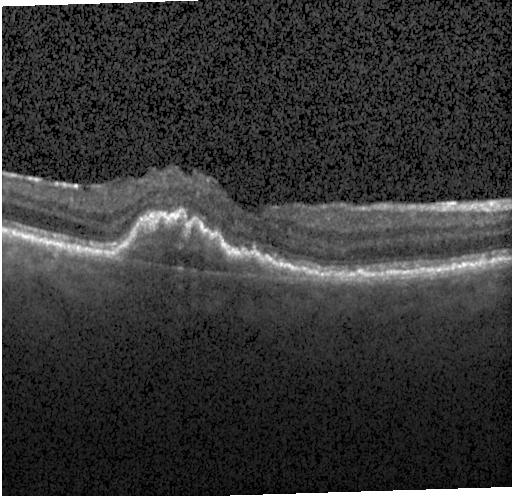 OCT scan showing choroidal neovascularization (CNV).